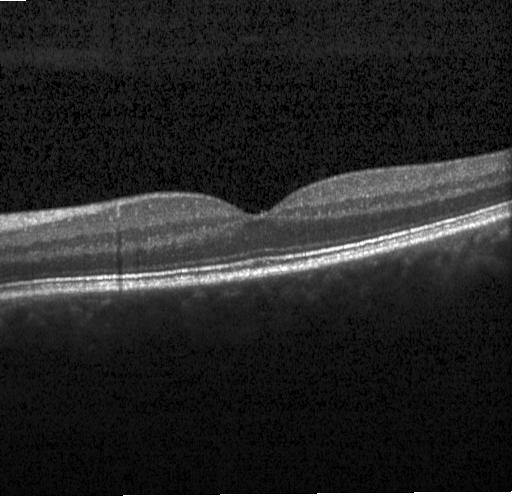
OCT line scan
Macular OCT: no choroidal neovascularization, diabetic macular edema, or drusen.